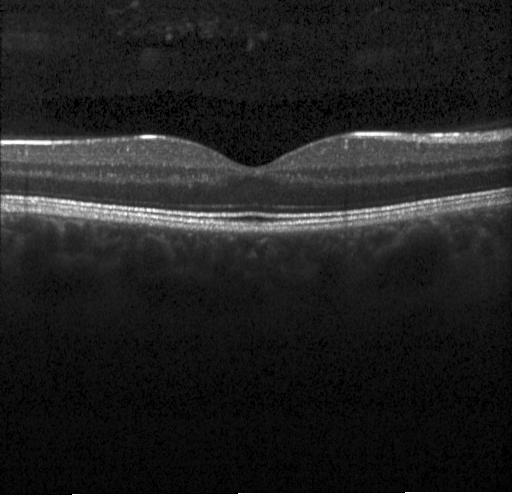
Fovea-centered, Heidelberg Spectralis OCT system, retinal OCT cross-section
Macular OCT: no evidence of CNV, DME, or drusen.